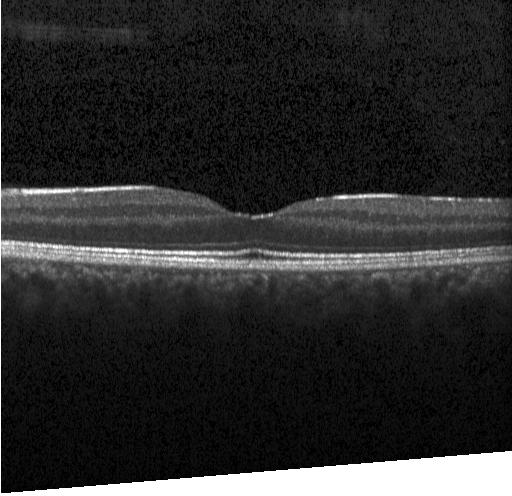 Through the macula. Acquired on a Heidelberg Spectralis. OCT B-scan. Impression: no CNV, no DME, and no drusen.